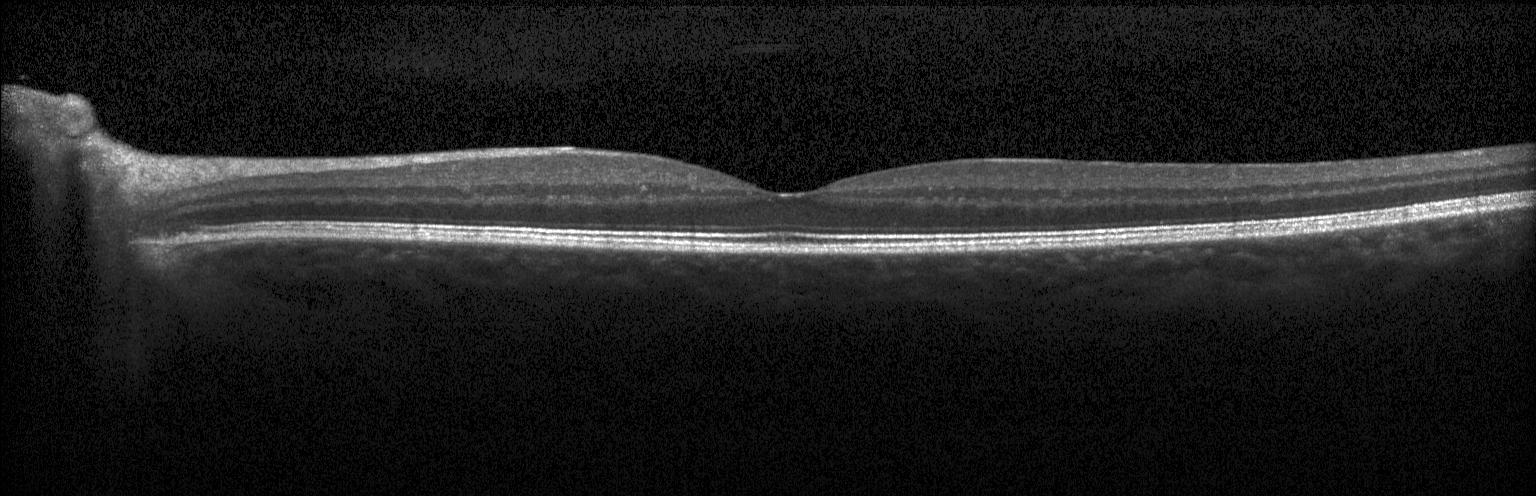 Macular OCT demonstrating no choroidal neovascularization, diabetic macular edema, or drusen.